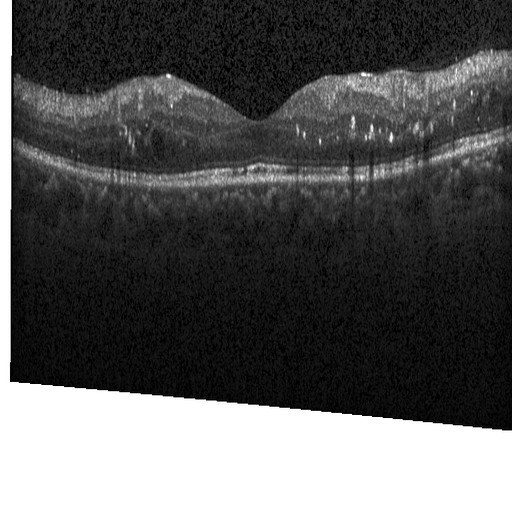 Retinal OCT cross-section — Impression: DME.